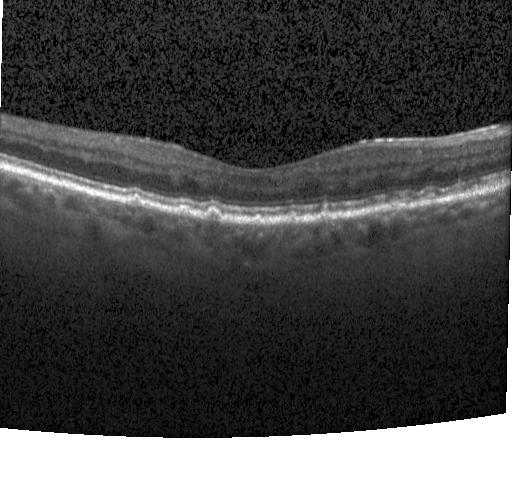
Spectral-domain OCT B-scan: sub-RPE drusenoid deposits.